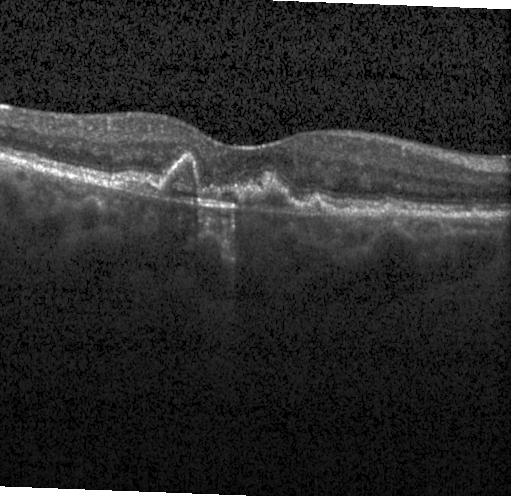 Impression: a choroidal neovascular membrane.